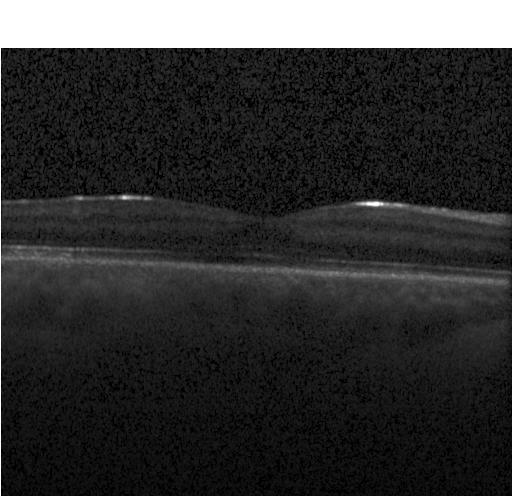 Macular OCT: no choroidal neovascularization, no diabetic macular edema, and no drusen.